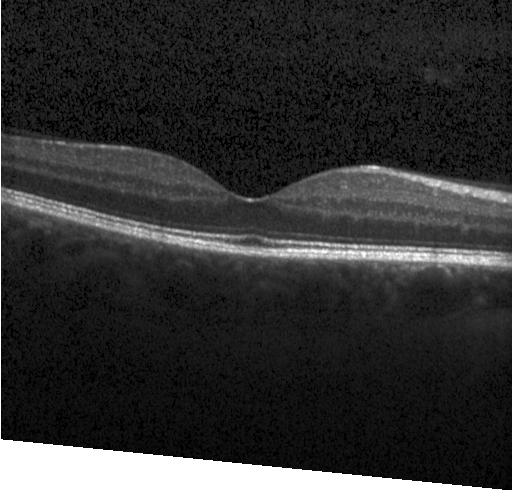

Fovea-centered · retinal OCT B-scan.
Macular OCT: neither choroidal neovascularization, diabetic macular edema, nor drusen.